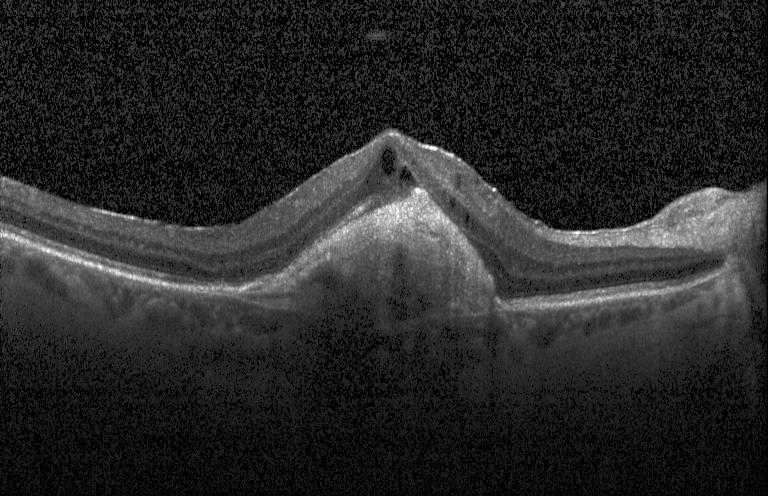
Optical coherence tomography scan — Impression: a choroidal neovascular membrane.